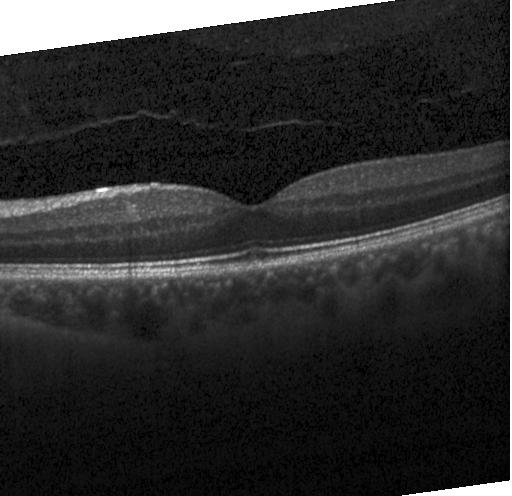

Finding: neither CNV, DME, nor drusen.